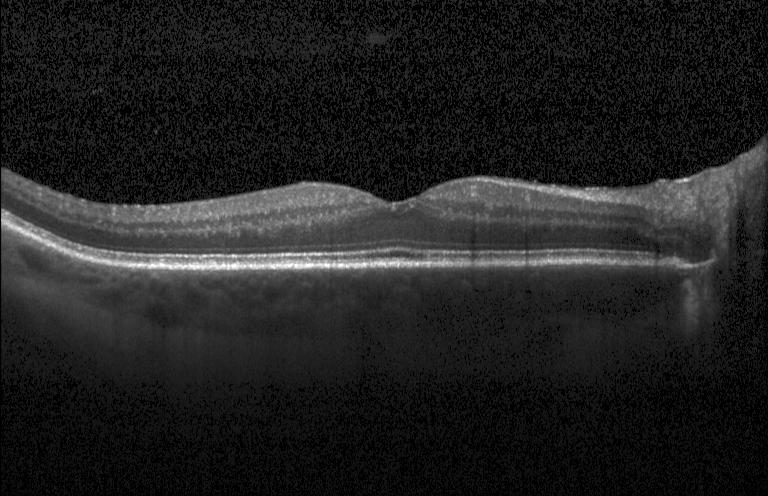

Retinal OCT cross-section; instrument: Heidelberg Spectralis — Assessment: no evidence of choroidal neovascularization, diabetic macular edema, or drusen.